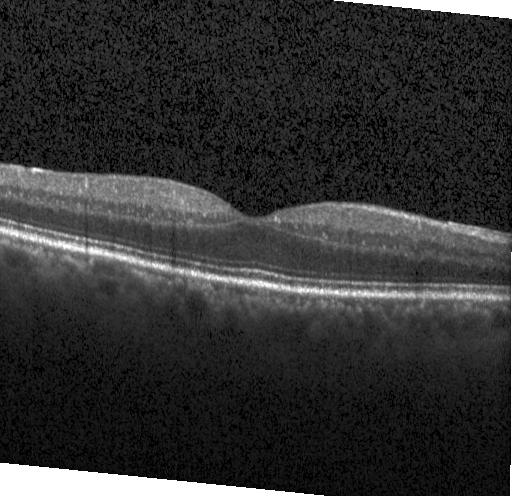

Centered on the fovea, spectral-domain OCT, retinal OCT B-scan. Diagnosis: neither choroidal neovascularization, diabetic macular edema, nor drusen.